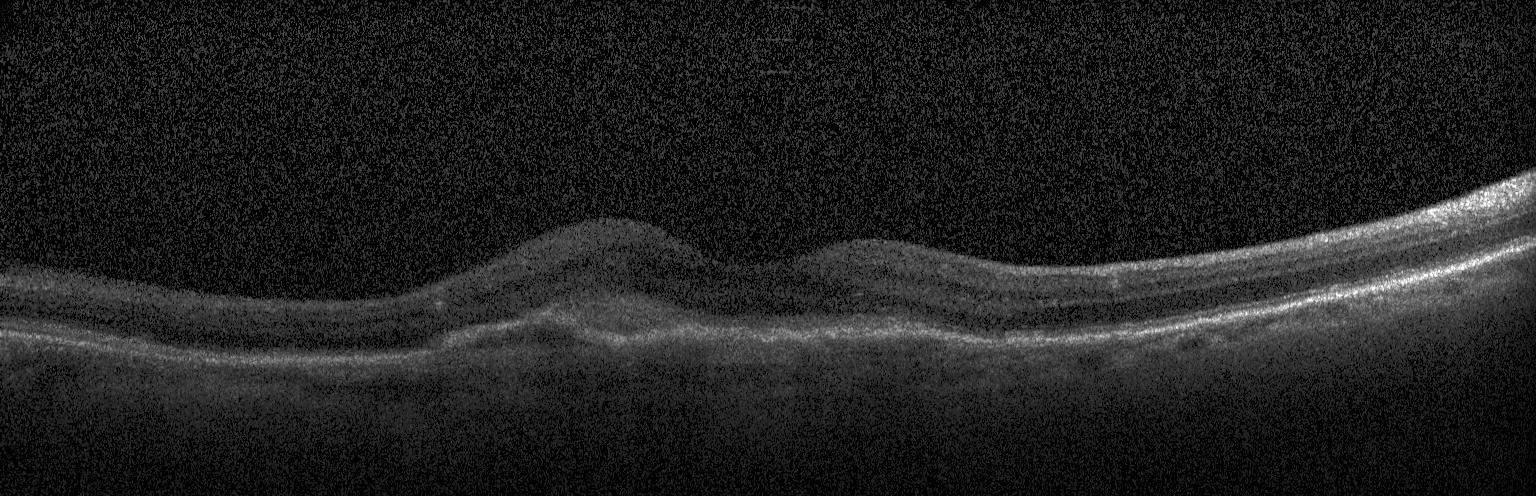

OCT B-scan; macular scan. Assessment: a choroidal neovascular membrane.